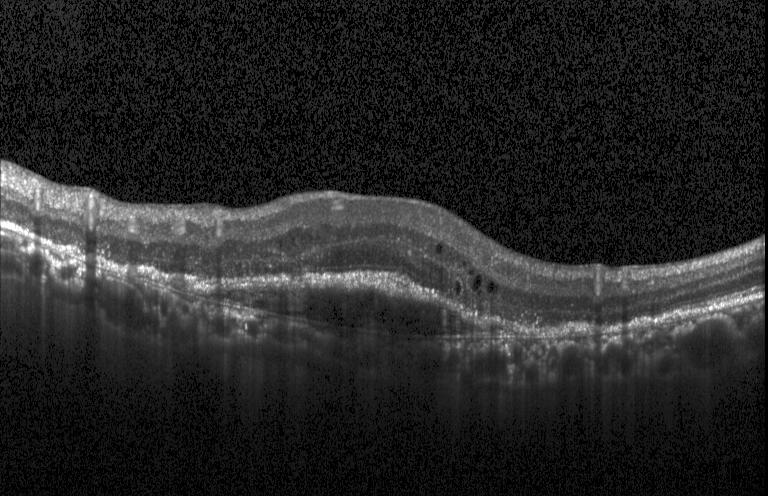 Diagnosis: a choroidal neovascular membrane.